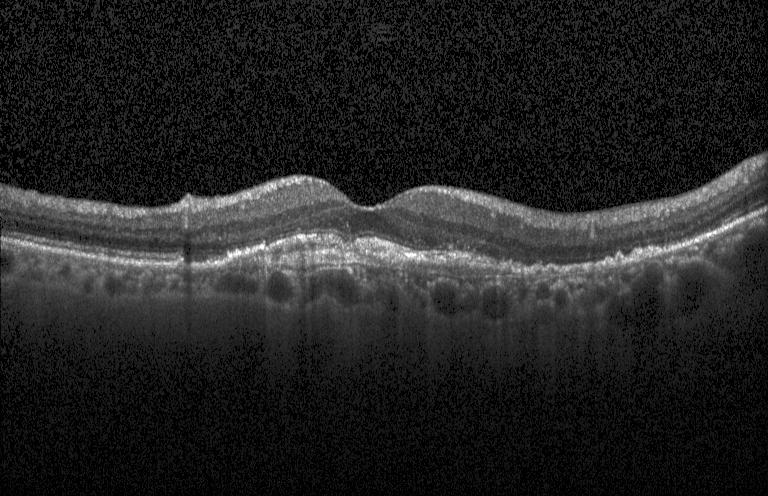 Macular OCT demonstrating a choroidal neovascular membrane.